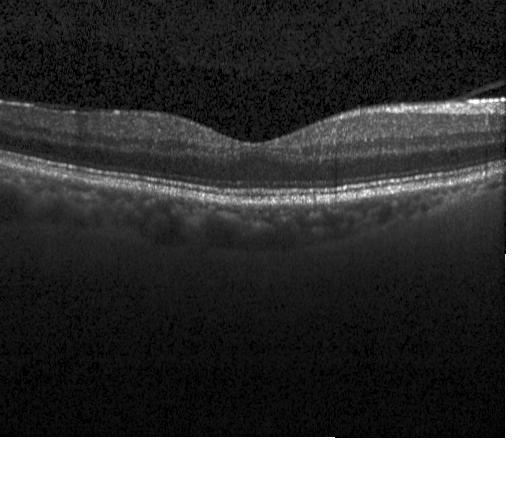
Retinal OCT cross-section. Heidelberg Spectralis OCT system. Macular scan. Assessment: no choroidal neovascularization, diabetic macular edema, or drusen.